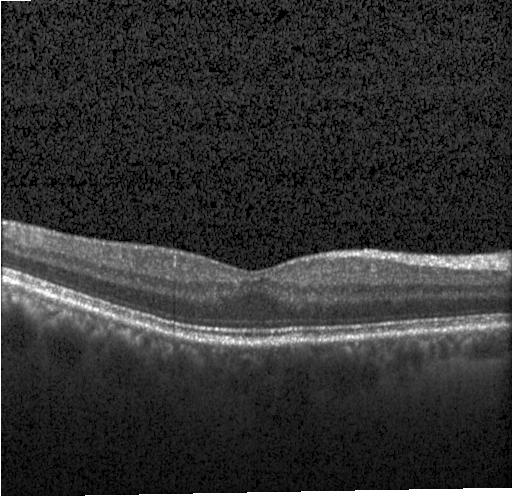 No choroidal neovascularization, no diabetic macular edema, and no drusen.